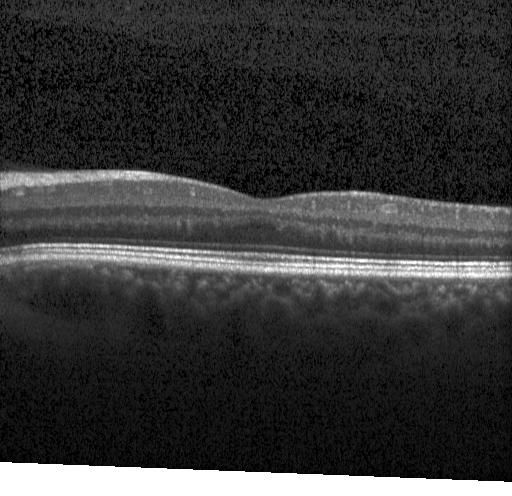
Acquired on a Heidelberg Spectralis · spectral-domain optical coherence tomography · optical coherence tomography scan · through the macula — OCT finding: no evidence of choroidal neovascularization, diabetic macular edema, or drusen.